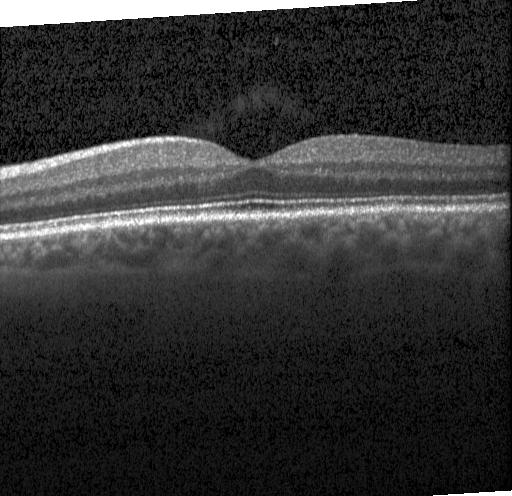 Optical coherence tomography scan. Macular OCT: no evidence of choroidal neovascularization, diabetic macular edema, or drusen.